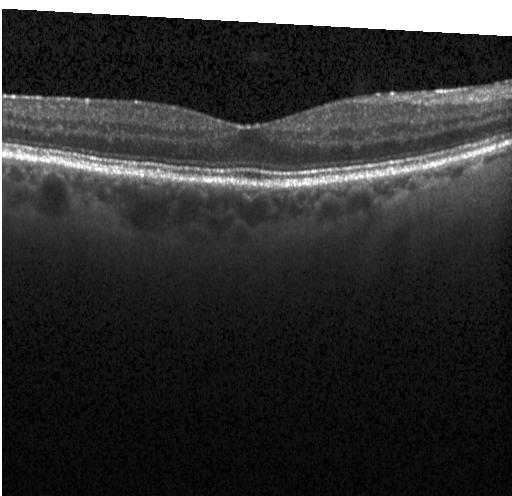
OCT B-scan
Finding: no CNV, no DME, and no drusen.